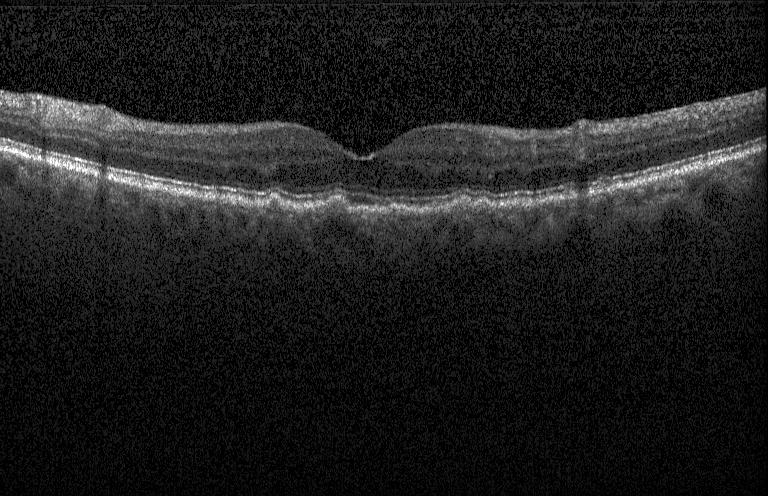
Macular OCT demonstrating sub-RPE drusenoid deposits.